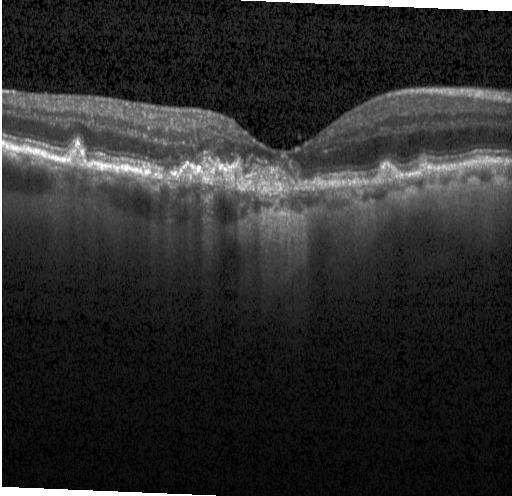 Optical coherence tomography scan; acquired on a Heidelberg Spectralis
Assessment: choroidal neovascularization.